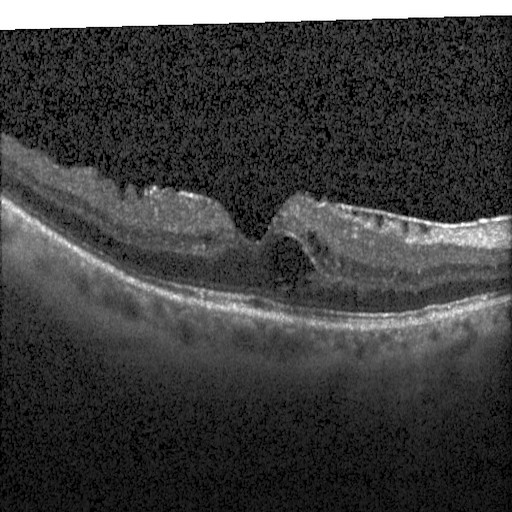

SD-OCT. OCT line scan
Assessment: diabetic macular edema.